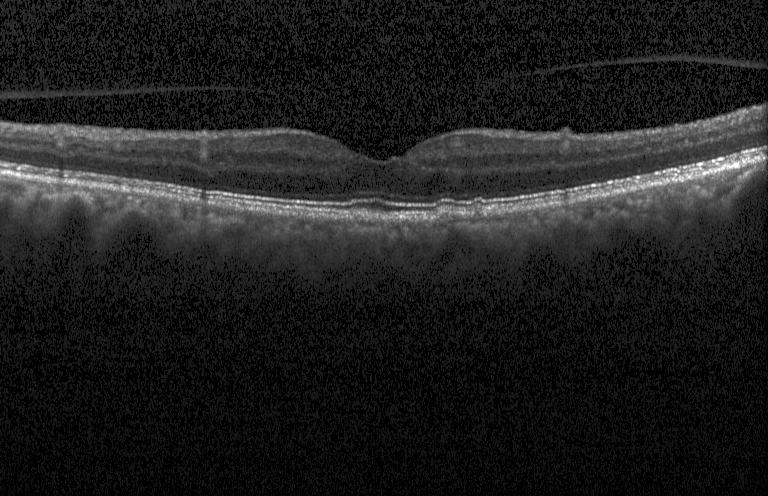 Horizontal scan through the fovea. Heidelberg Spectralis OCT system. Optical coherence tomography scan. SD-OCT
Diagnosis: multiple drusen.